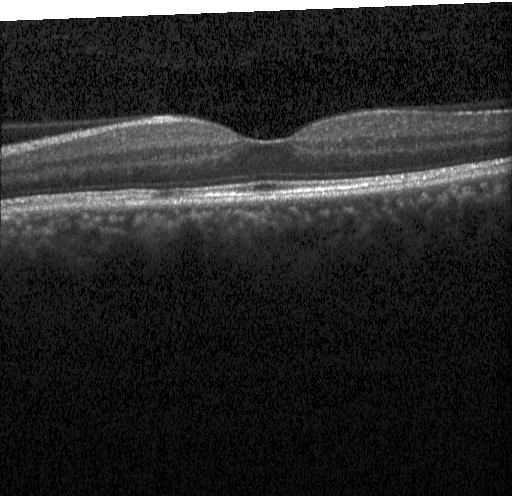 The scan shows no evidence of choroidal neovascularization, diabetic macular edema, or drusen.